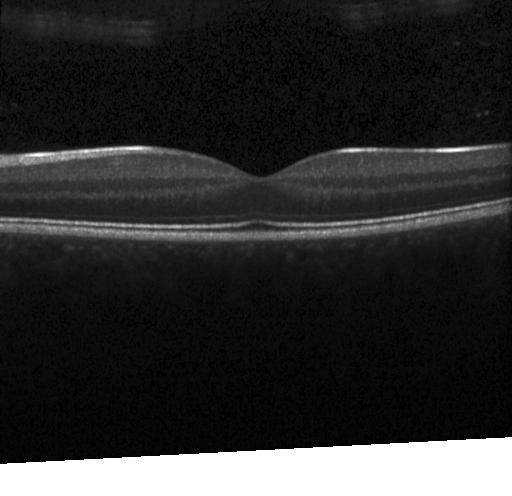
This B-scan demonstrates no choroidal neovascularization, no diabetic macular edema, and no drusen.